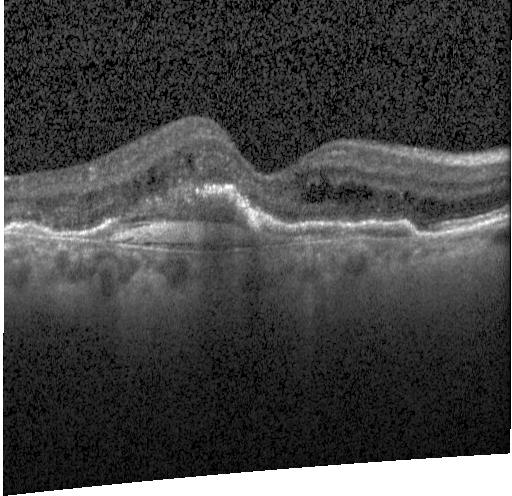
Spectral-domain OCT; instrument: Heidelberg Spectralis; through the macula; optical coherence tomography B-scan — Impression: choroidal neovascularization (CNV).